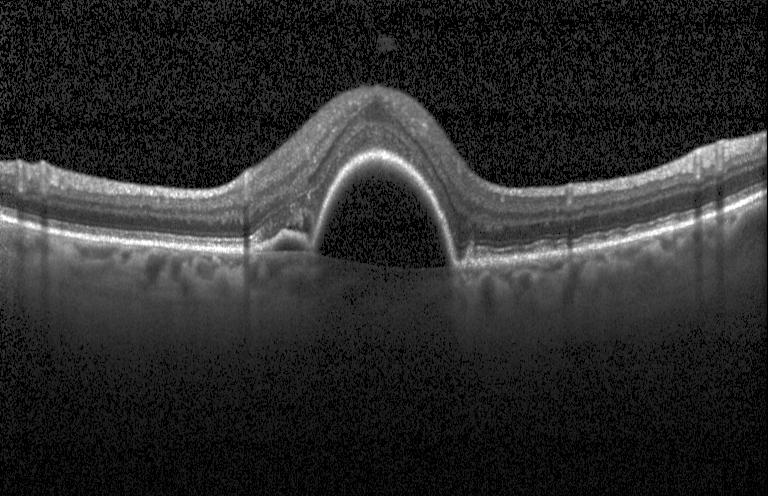 The scan shows a choroidal neovascular membrane.